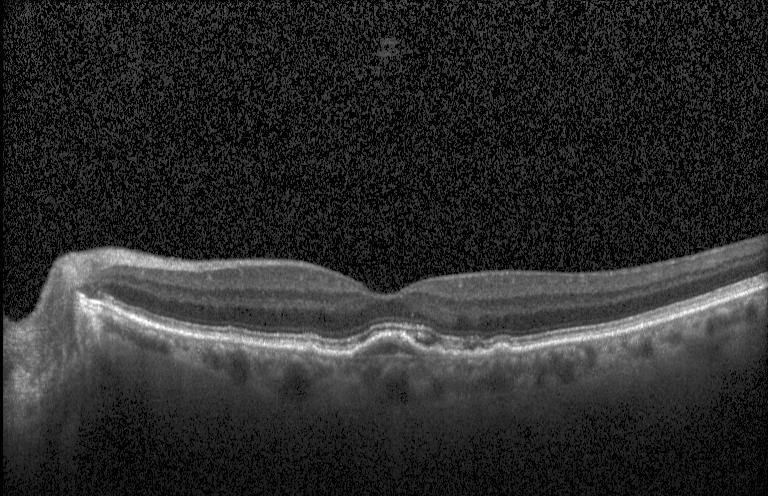 Optical coherence tomography scan; instrument: Heidelberg Spectralis; spectral-domain OCT; macular scan. Impression: CNV.